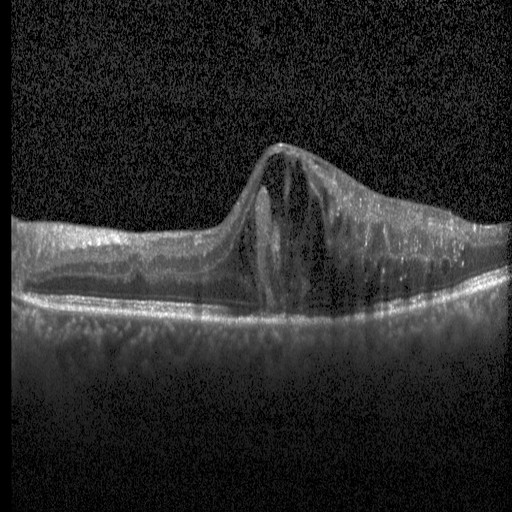
Centered on the fovea. Spectral-domain optical coherence tomography. OCT line scan
Finding: diabetic macular edema.